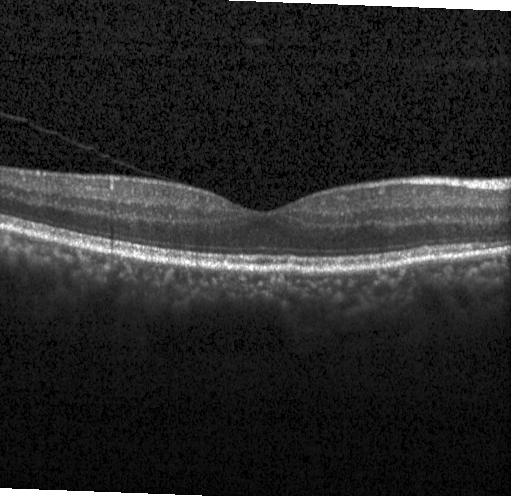

Assessment: no choroidal neovascularization, diabetic macular edema, or drusen.